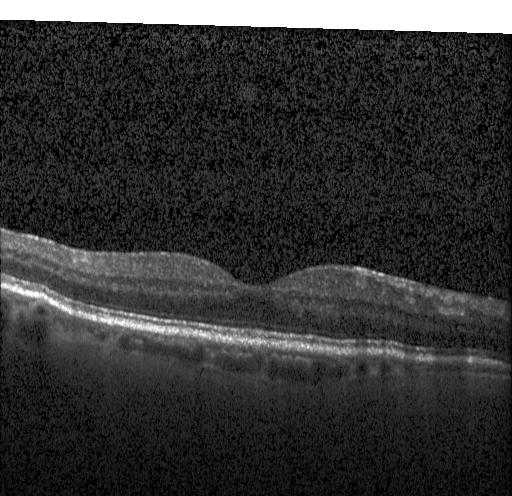 Retinal OCT B-scan. Diagnosis: neither choroidal neovascularization, diabetic macular edema, nor drusen.